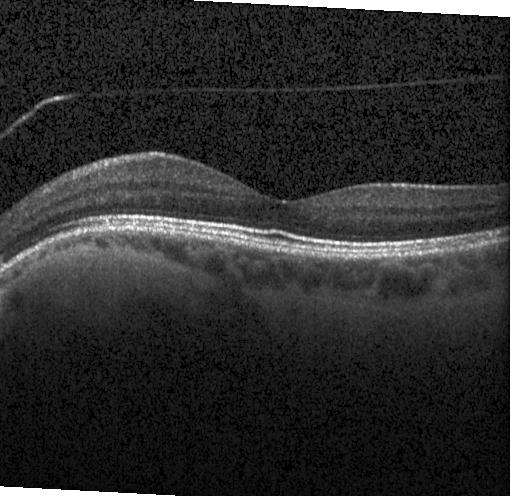 No choroidal neovascularization, no diabetic macular edema, and no drusen.